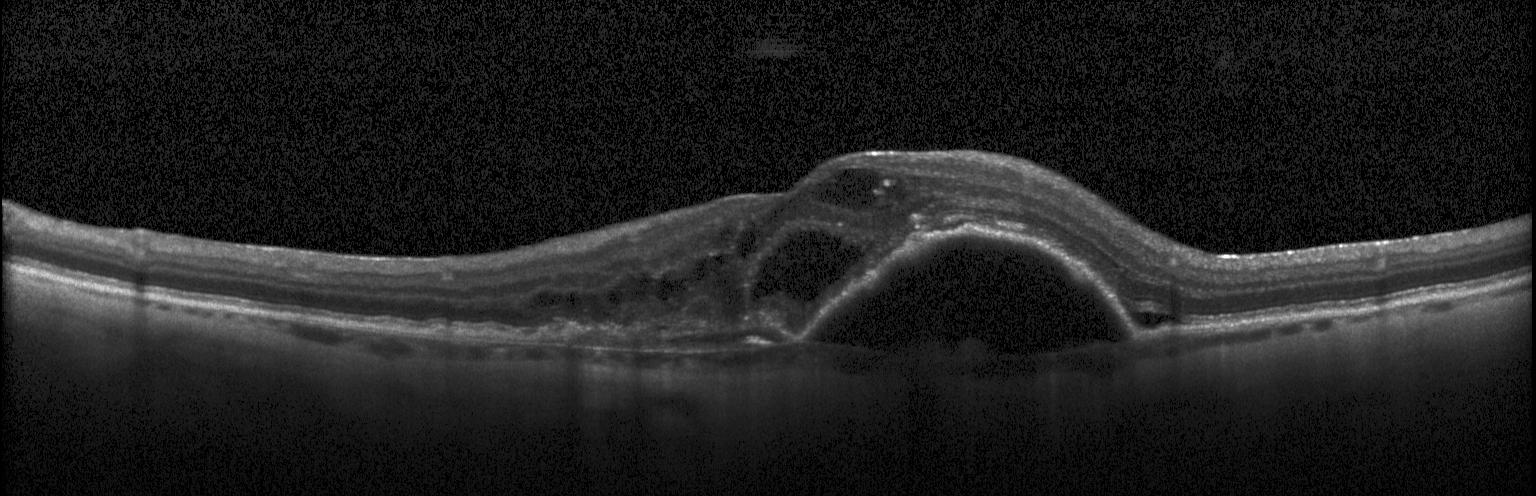

Diagnosis: choroidal neovascularization (CNV).